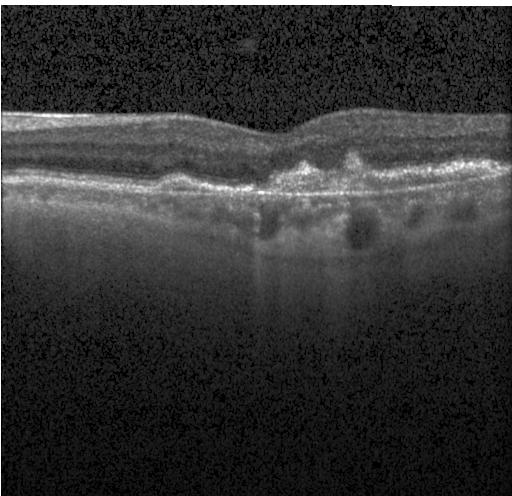
This B-scan demonstrates a choroidal neovascular membrane.